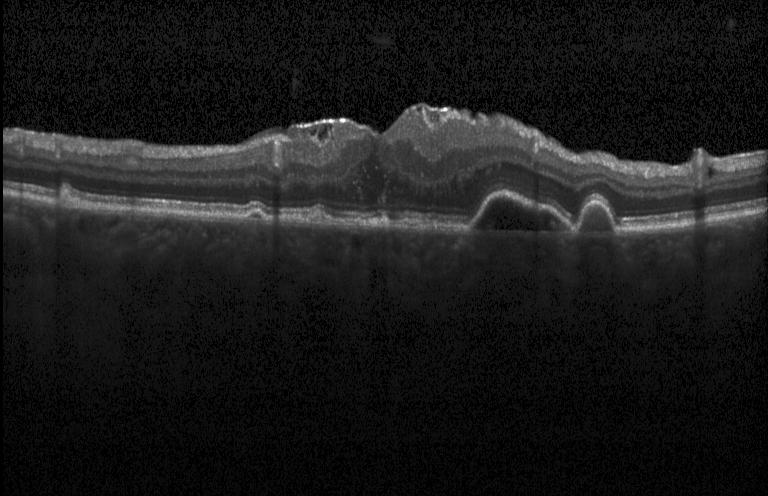 Dx: a choroidal neovascular membrane.